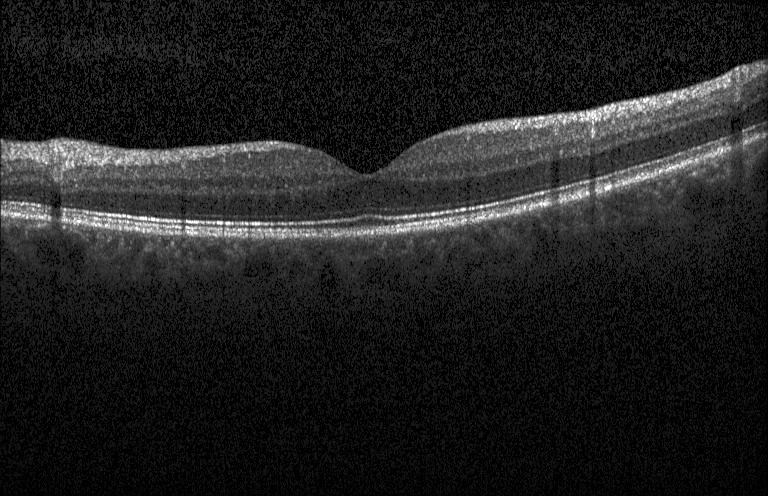 Retinal OCT cross-section showing no evidence of choroidal neovascularization, diabetic macular edema, or drusen.